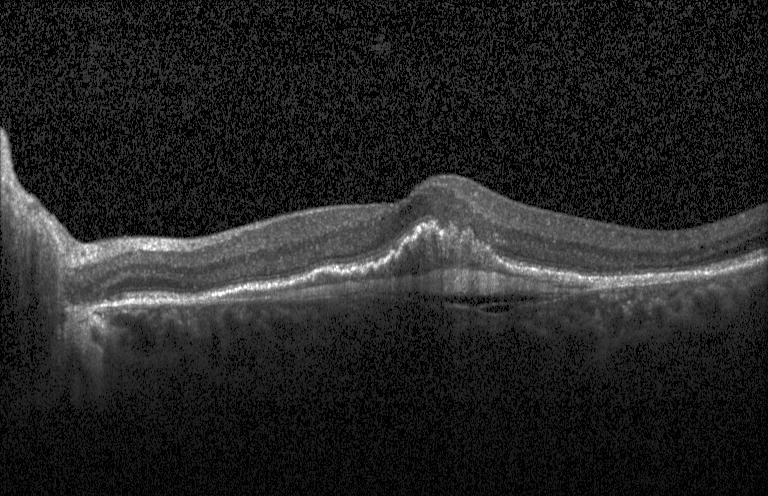
Diagnosis: a choroidal neovascular membrane.